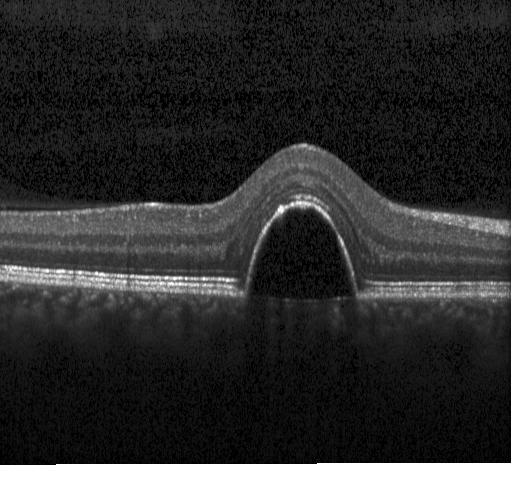

Retinal OCT cross-section — This B-scan demonstrates a choroidal neovascular membrane.